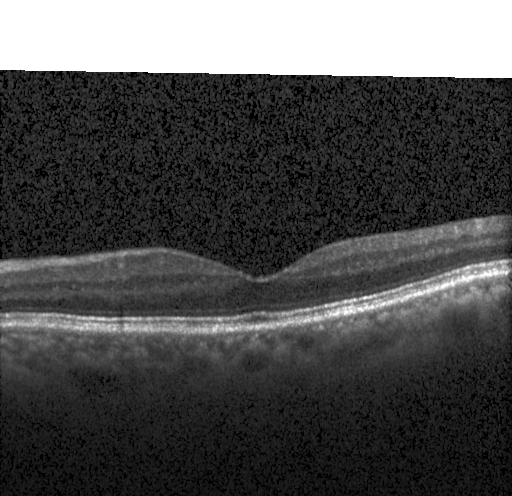
OCT finding: no CNV, DME, or drusen.